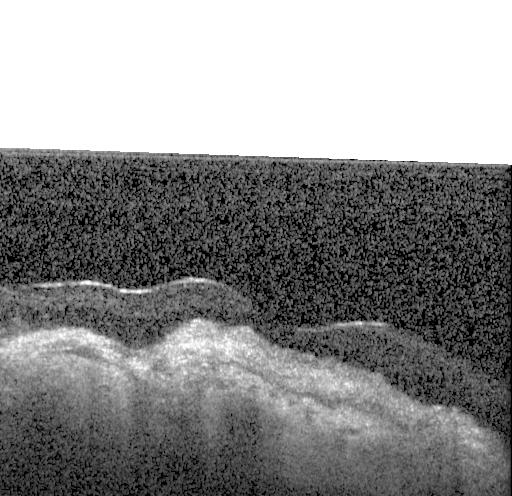 Retinal OCT B-scan, instrument: Heidelberg Spectralis
Impression: a choroidal neovascular membrane.